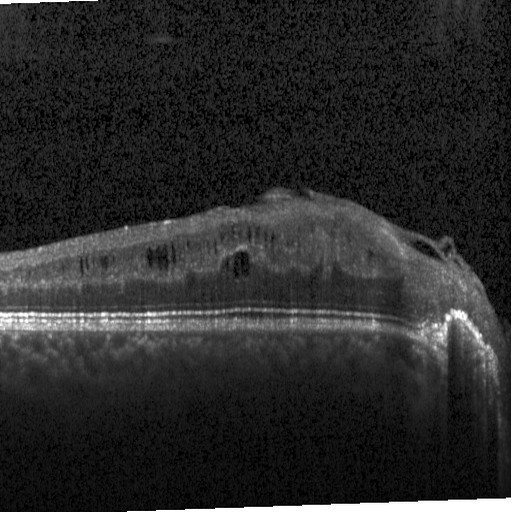 Macular scan, OCT line scan, spectral-domain optical coherence tomography.
Finding: diabetic macular edema.